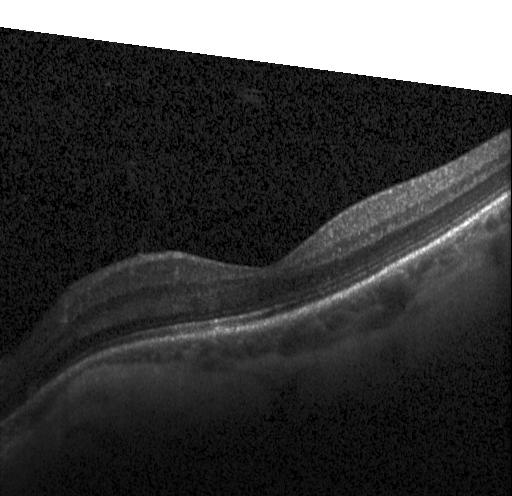
Finding: no choroidal neovascularization, no diabetic macular edema, and no drusen.